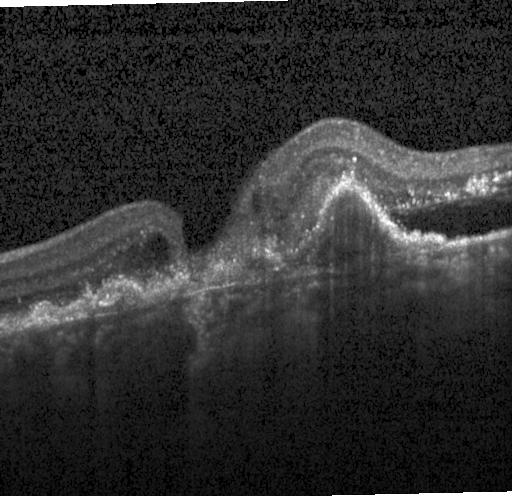 Retinal OCT cross-section, through the macula, spectral-domain OCT, Heidelberg Spectralis — Finding: a choroidal neovascular membrane.